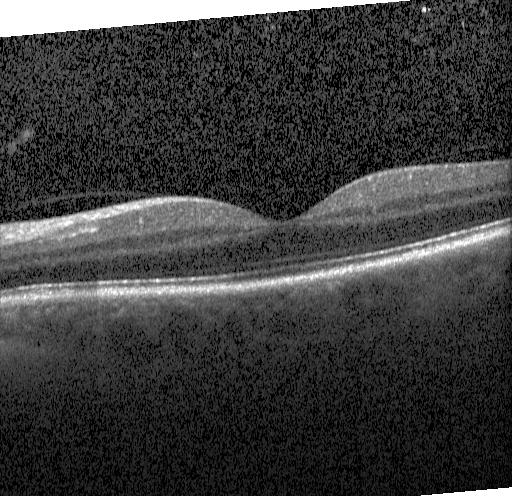
Macular OCT: neither CNV, DME, nor drusen.